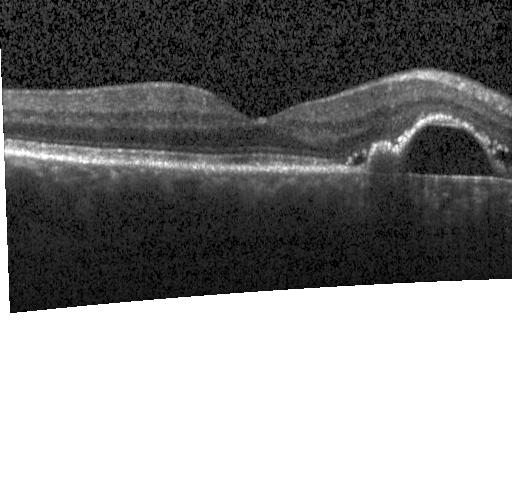
Retinal OCT B-scan, instrument: Heidelberg Spectralis, horizontal scan through the fovea, spectral-domain OCT. Dx: choroidal neovascularization.